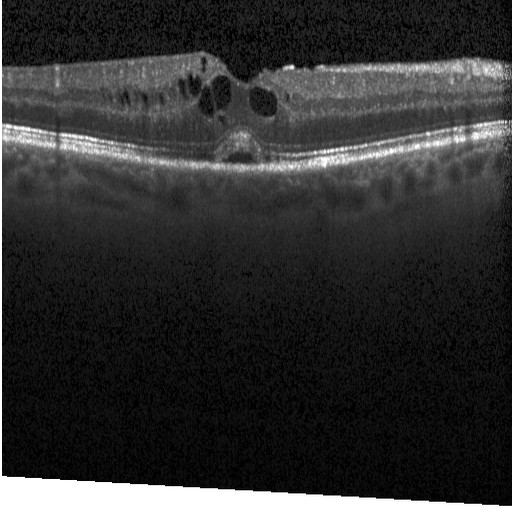 DME.